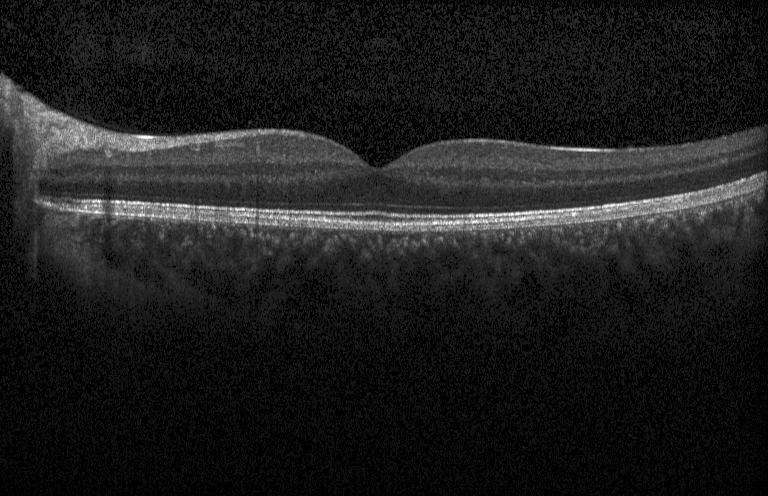 Retinal OCT cross-section showing no CNV, no DME, and no drusen.